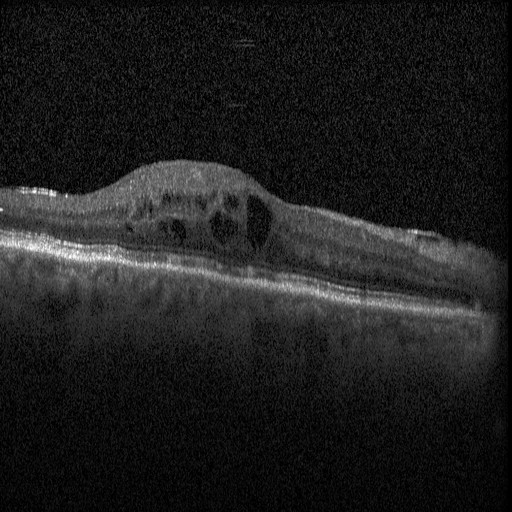

OCT line scan
Impression: DME.